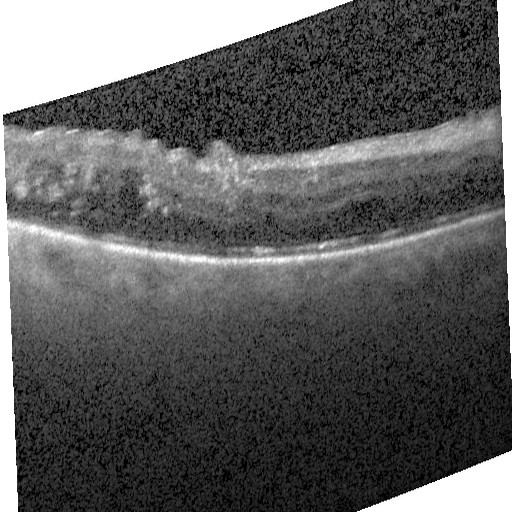
OCT B-scan, through the macula, acquired on a Heidelberg Spectralis — Finding: diabetic macular edema.